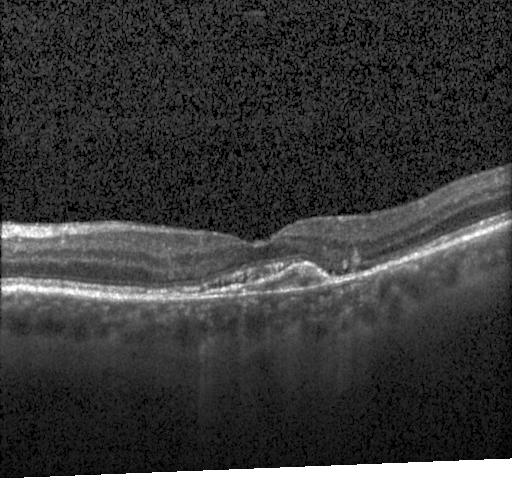 Instrument: Heidelberg Spectralis; OCT B-scan
Diagnosis: a choroidal neovascular membrane.